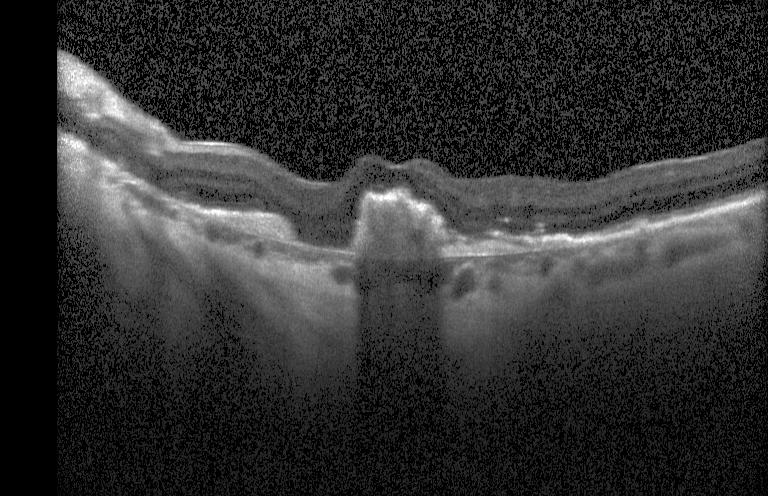
Macular OCT demonstrating a choroidal neovascular membrane.